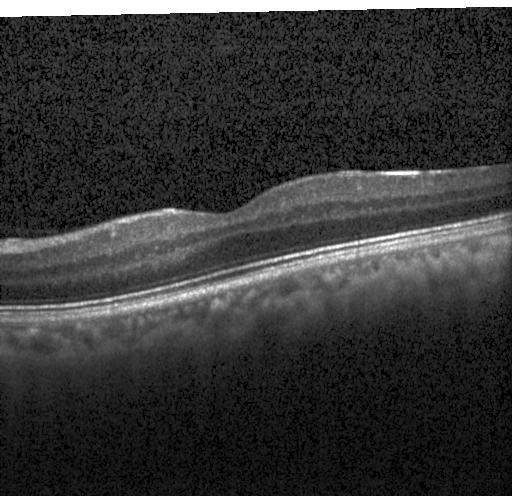 SD-OCT, retinal OCT cross-section, instrument: Heidelberg Spectralis, through the macula
Diagnosis: no CNV, no DME, and no drusen.